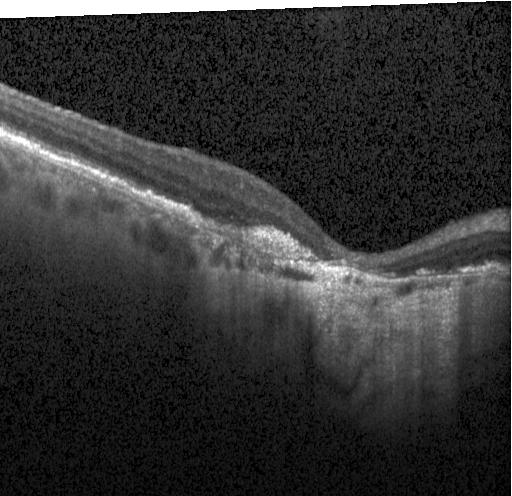 Optical coherence tomography B-scan; instrument: Heidelberg Spectralis; fovea-centered. Dx: a choroidal neovascular membrane.